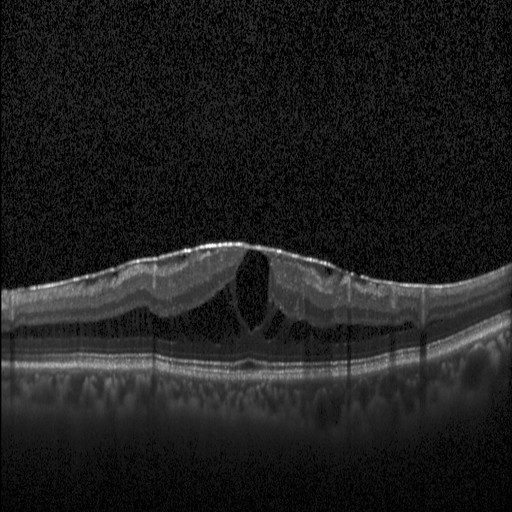

Impression: diabetic macular edema.